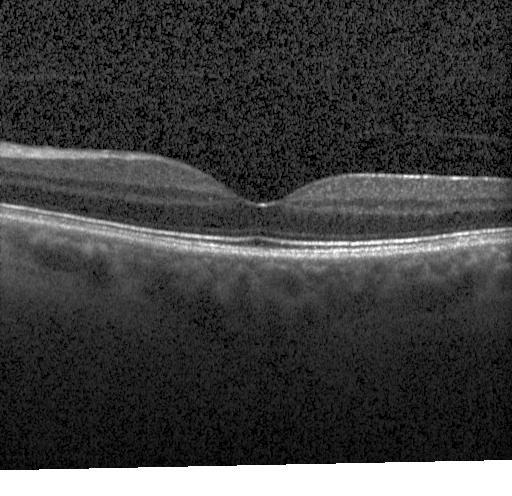
OCT B-scan. Macular scan — Diagnosis: no CNV, DME, or drusen.